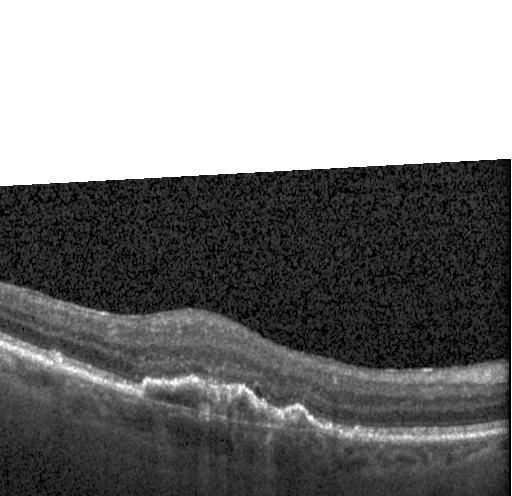

Macular scan. Optical coherence tomography scan
Impression: a choroidal neovascular membrane.